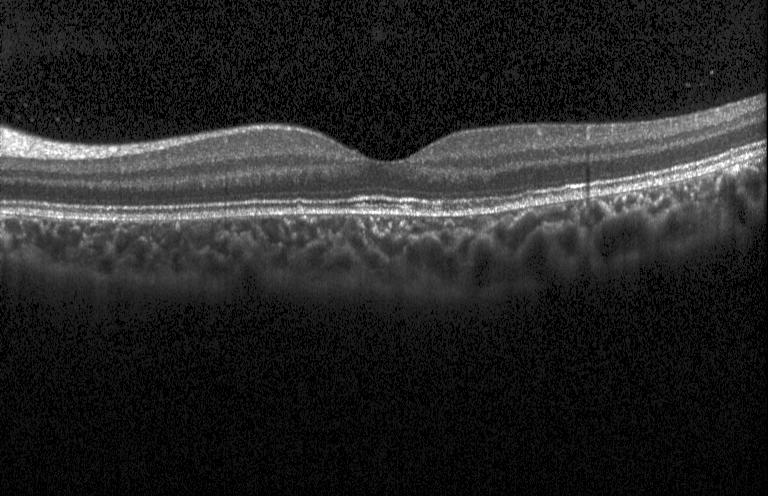
Dx: no choroidal neovascularization, diabetic macular edema, or drusen.